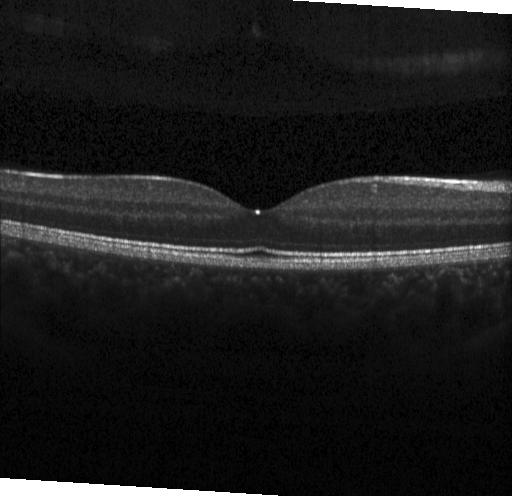
Retinal OCT B-scan. Diagnosis: no CNV, no DME, and no drusen.